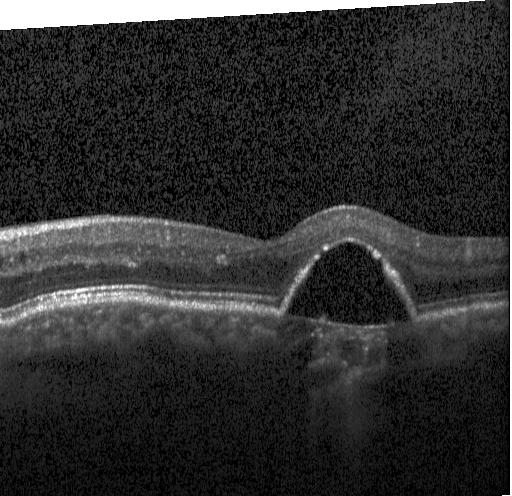 Fovea-centered, Heidelberg Spectralis, retinal OCT cross-section. Assessment: a choroidal neovascular membrane.